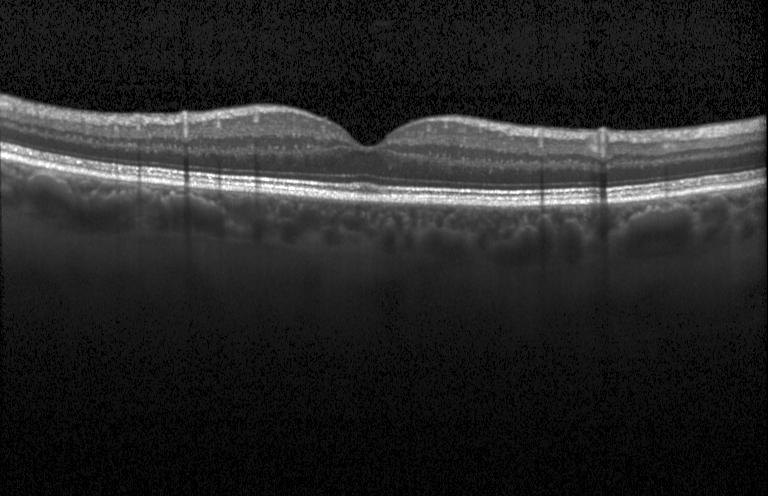

Macular scan, OCT B-scan — OCT finding: neither choroidal neovascularization, diabetic macular edema, nor drusen.